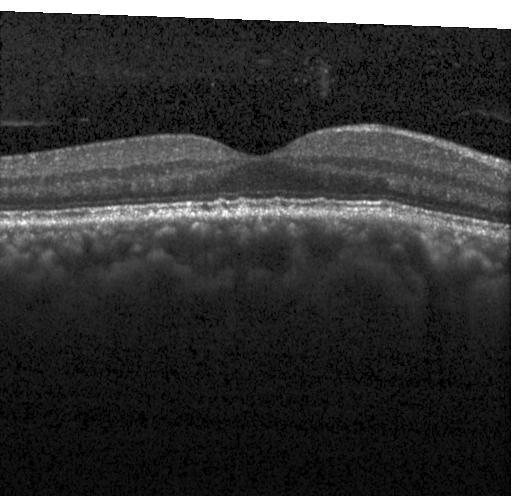

OCT scan showing multiple drusen.